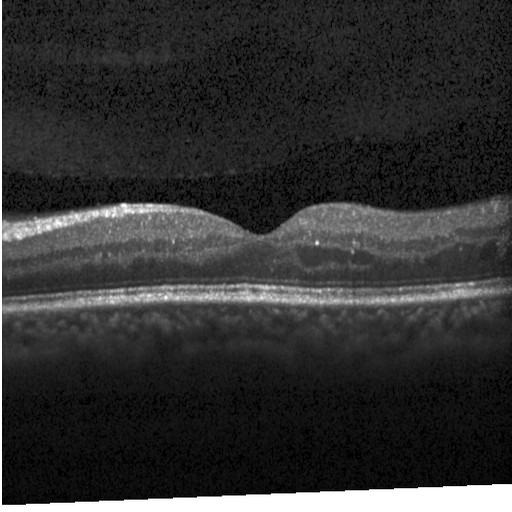
Through the macula · OCT B-scan. Finding: diabetic macular edema.